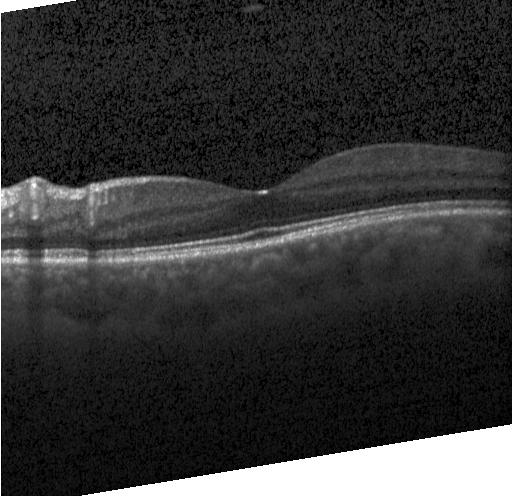
Macular scan · retinal OCT B-scan · Heidelberg Spectralis — Assessment: no evidence of choroidal neovascularization, diabetic macular edema, or drusen.